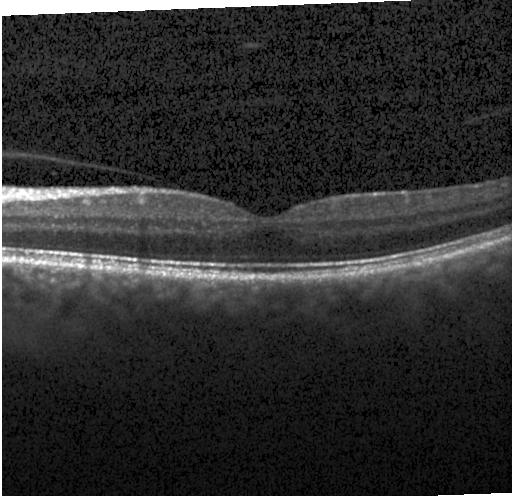 OCT finding: neither choroidal neovascularization, diabetic macular edema, nor drusen.